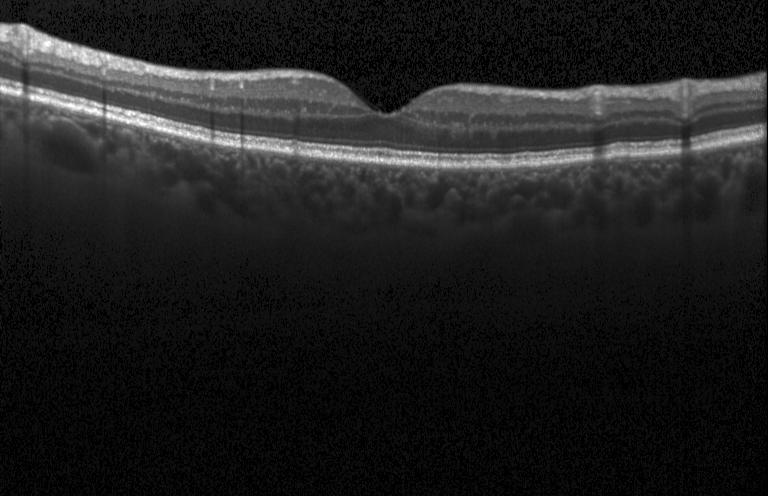 OCT line scan. Diagnosis: no choroidal neovascularization, no diabetic macular edema, and no drusen.